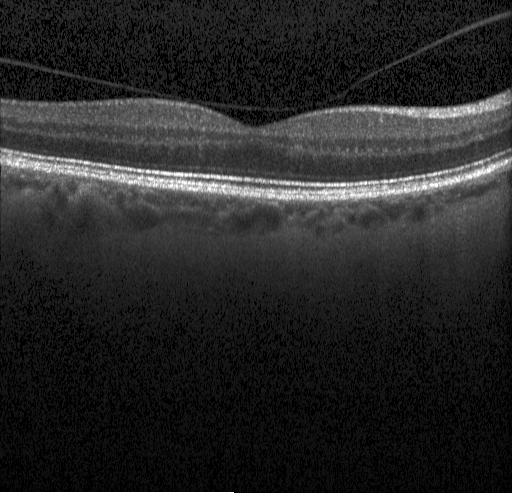 Instrument: Heidelberg Spectralis. Through the macula. Spectral-domain optical coherence tomography. Retinal OCT B-scan
This B-scan demonstrates no choroidal neovascularization, no diabetic macular edema, and no drusen.